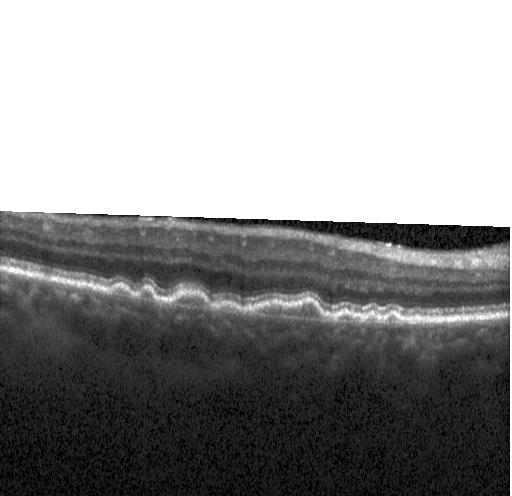

A choroidal neovascular membrane.